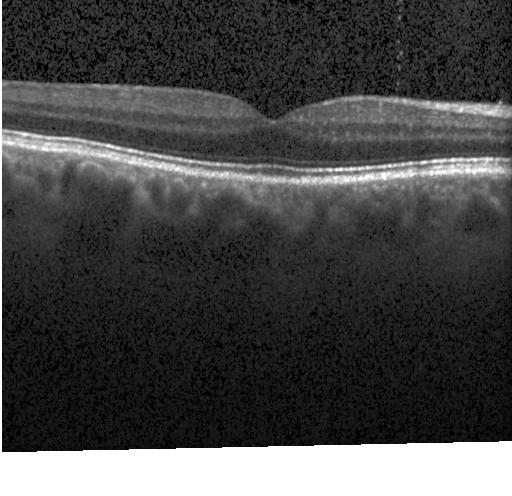 Impression: no choroidal neovascularization, no diabetic macular edema, and no drusen.